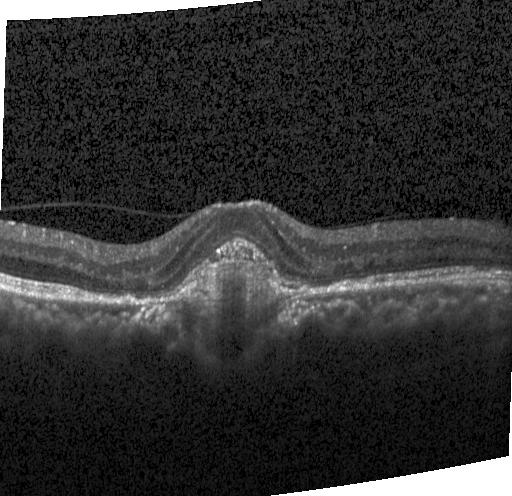

Dx: a choroidal neovascular membrane.